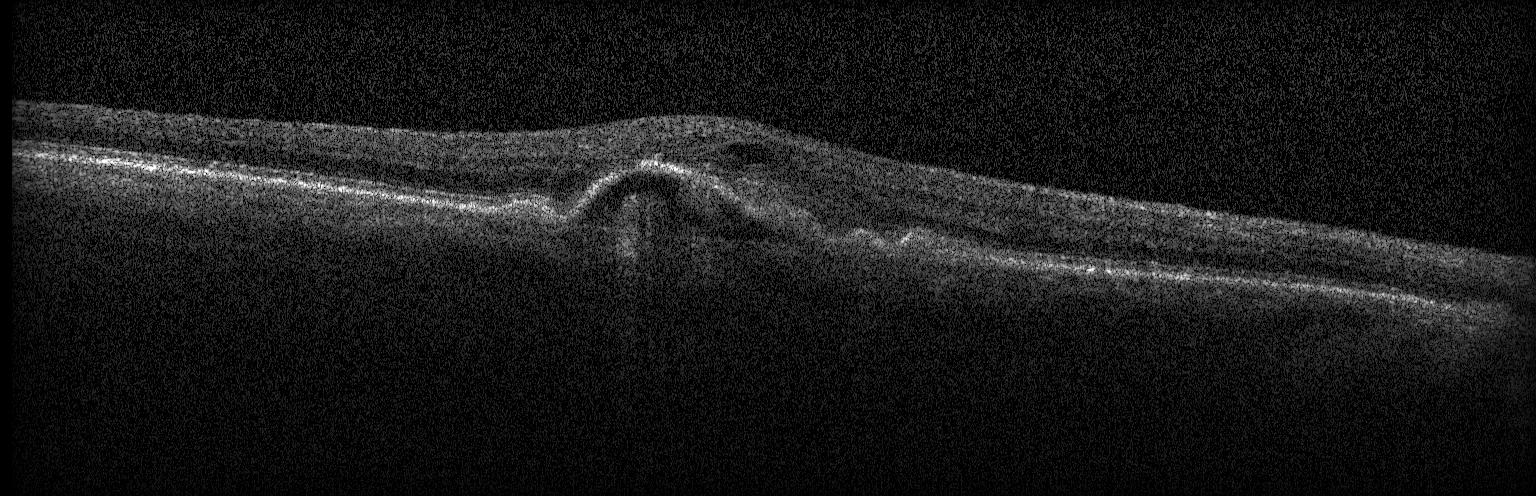
Macular OCT demonstrating a choroidal neovascular membrane.